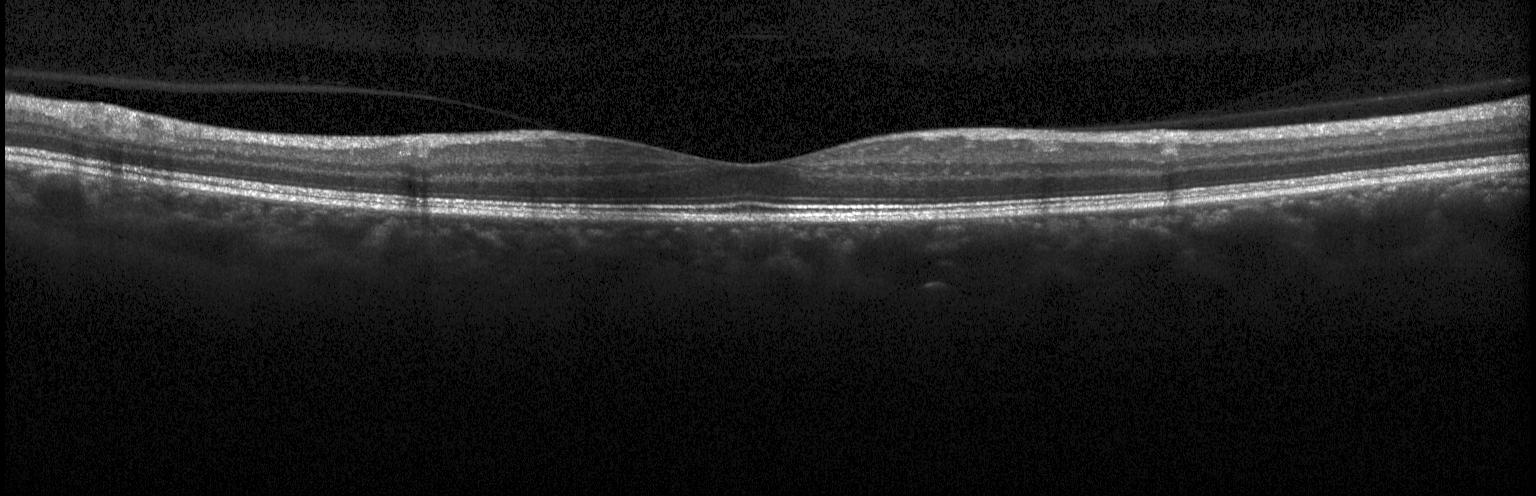
Retinal OCT B-scan — Impression: neither choroidal neovascularization, diabetic macular edema, nor drusen.